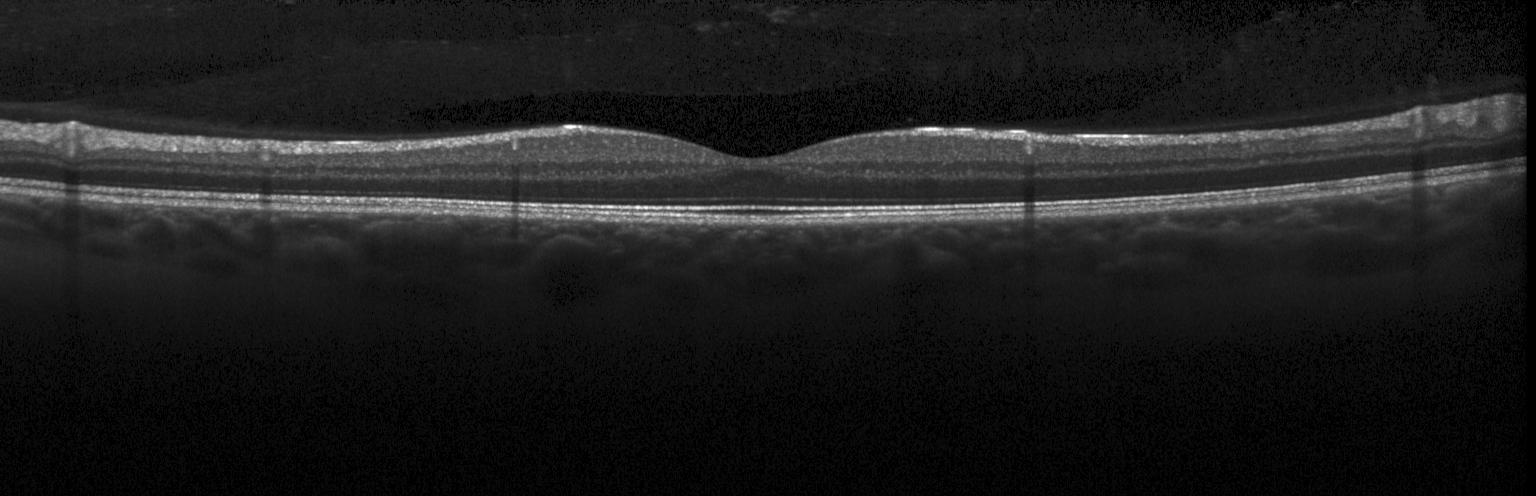

Optical coherence tomography B-scan, instrument: Heidelberg Spectralis, spectral-domain OCT. Finding: no choroidal neovascularization, diabetic macular edema, or drusen.